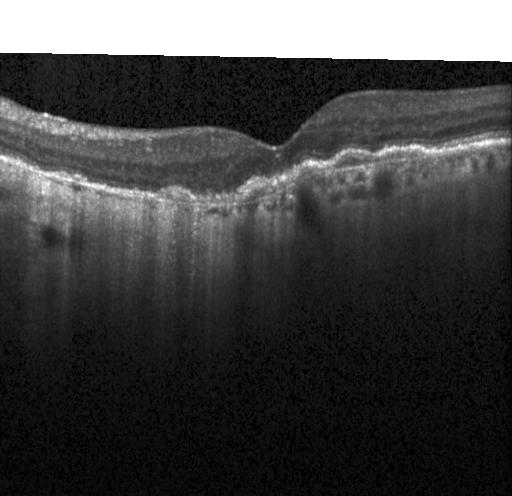

Acquired on a Heidelberg Spectralis; horizontal scan through the fovea; SD-OCT; retinal OCT cross-section — OCT finding: a choroidal neovascular membrane.